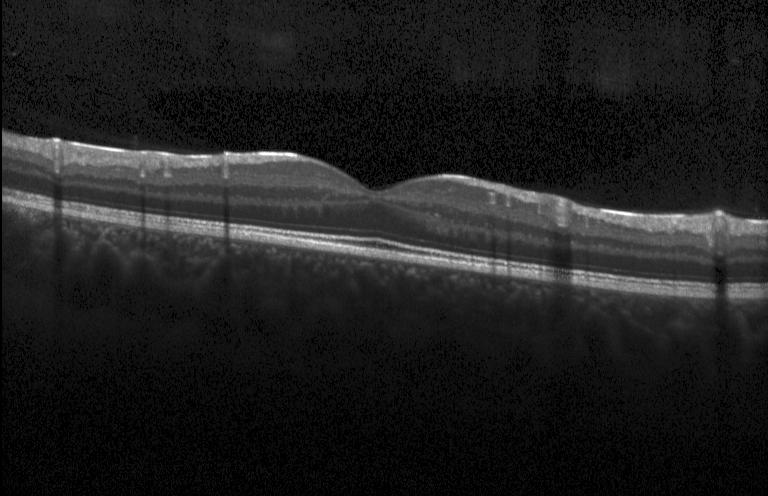

Heidelberg Spectralis · OCT line scan · horizontal scan through the fovea · spectral-domain OCT. Diagnosis: no CNV, no DME, and no drusen.